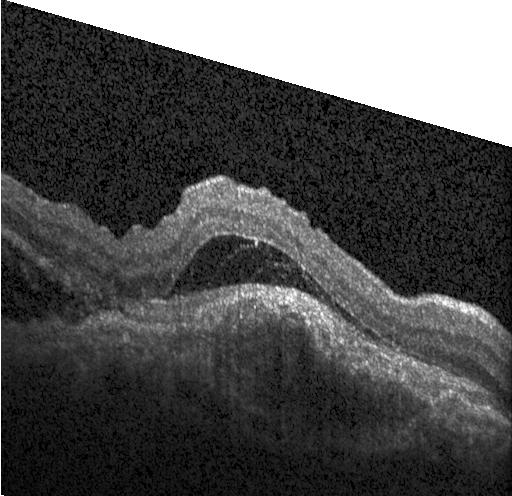 Macular scan · spectral-domain OCT · retinal OCT B-scan · acquired on a Heidelberg Spectralis. Finding: a choroidal neovascular membrane.